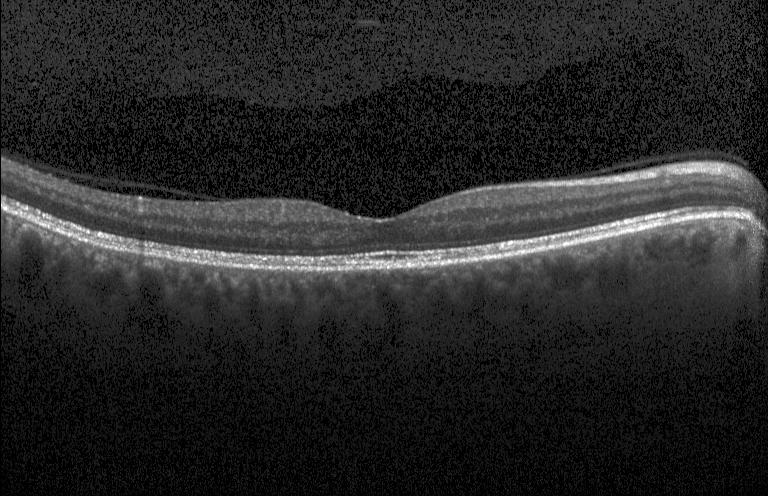

OCT scan showing no choroidal neovascularization, diabetic macular edema, or drusen.